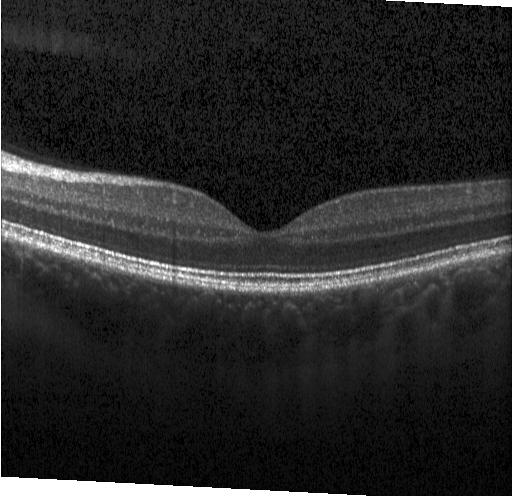

The scan shows no CNV, DME, or drusen.